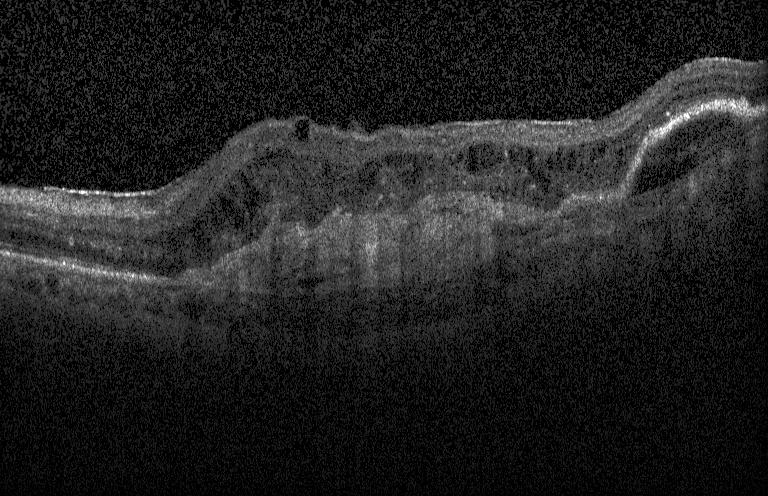

Diagnosis: a choroidal neovascular membrane.